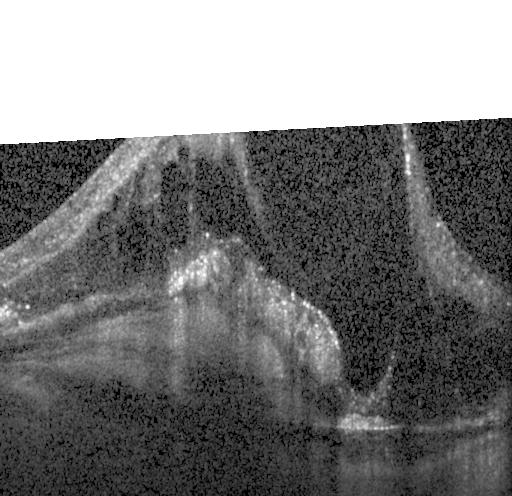

Spectral-domain OCT · retinal OCT cross-section — OCT finding: choroidal neovascularization.